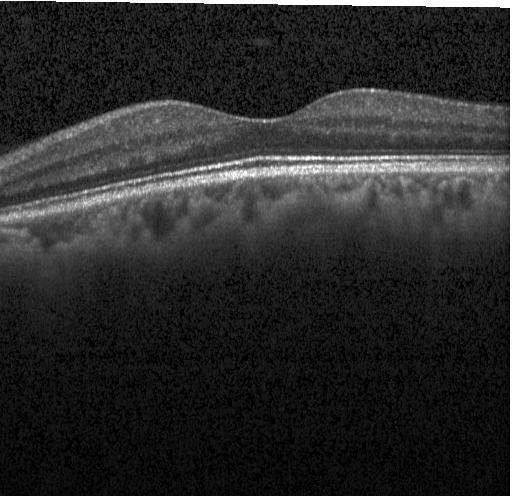 OCT finding: no evidence of choroidal neovascularization, diabetic macular edema, or drusen.